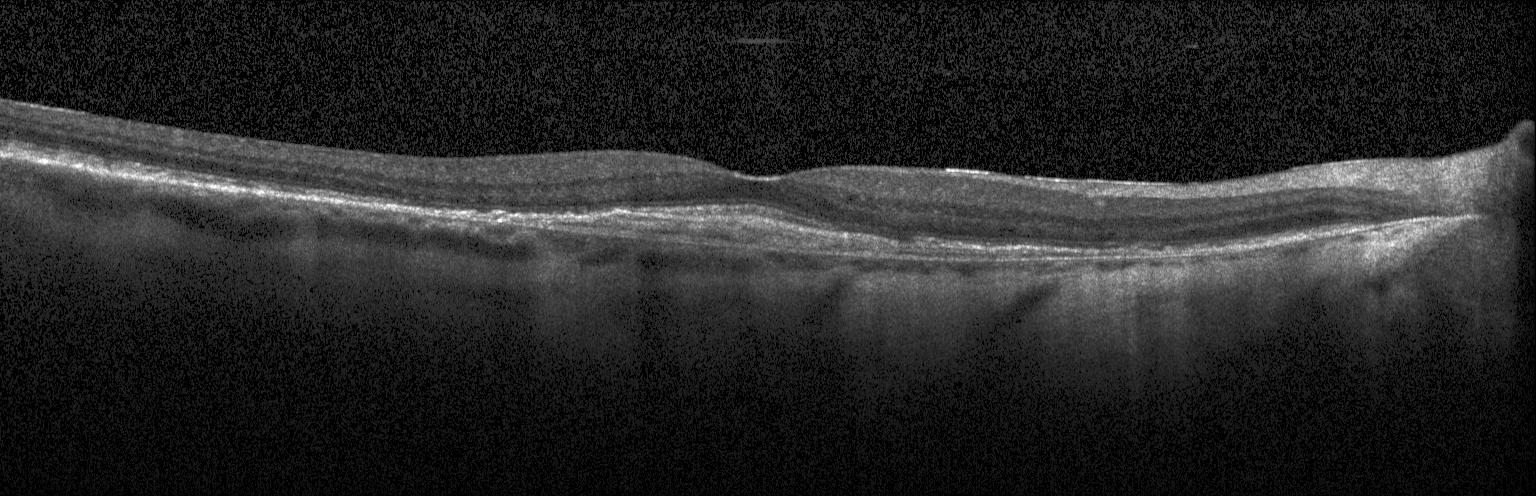

OCT line scan.
Macular OCT: a choroidal neovascular membrane.